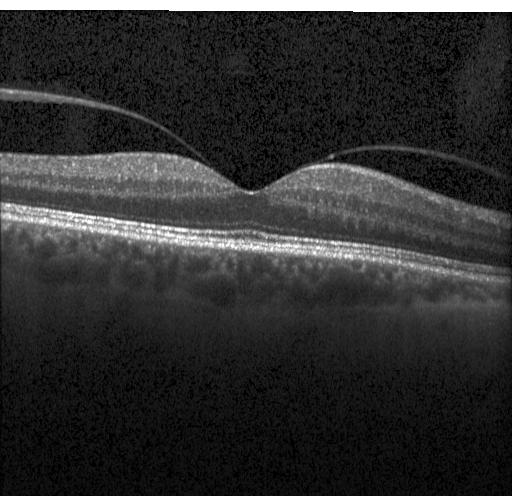

SD-OCT, OCT B-scan
Diagnosis: neither CNV, DME, nor drusen.